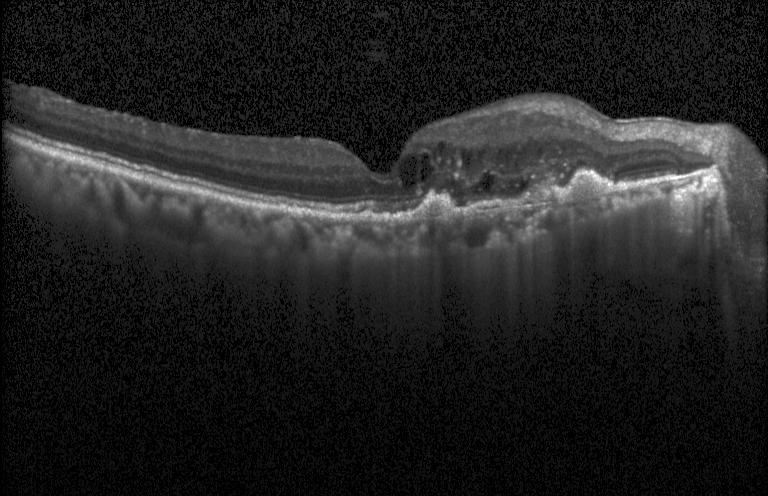 Optical coherence tomography B-scan. Fovea-centered. Acquired on a Heidelberg Spectralis. Spectral-domain optical coherence tomography — Assessment: choroidal neovascularization.